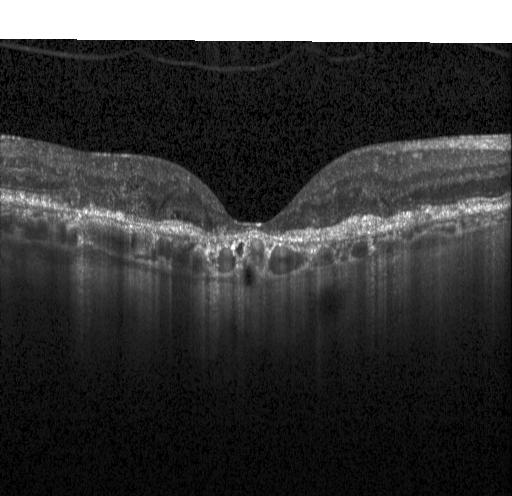

Spectral-domain optical coherence tomography; Heidelberg Spectralis; retinal OCT B-scan. Diagnosis: CNV.